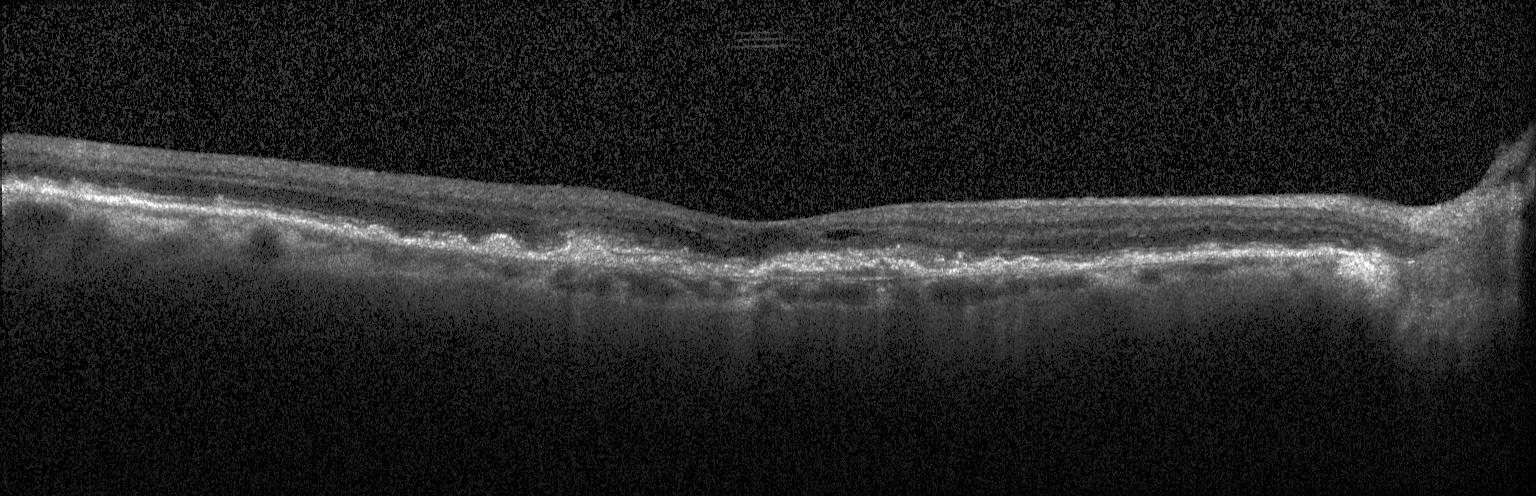
SD-OCT. Optical coherence tomography scan. Horizontal scan through the fovea. Acquired on a Heidelberg Spectralis — Diagnosis: choroidal neovascularization (CNV).